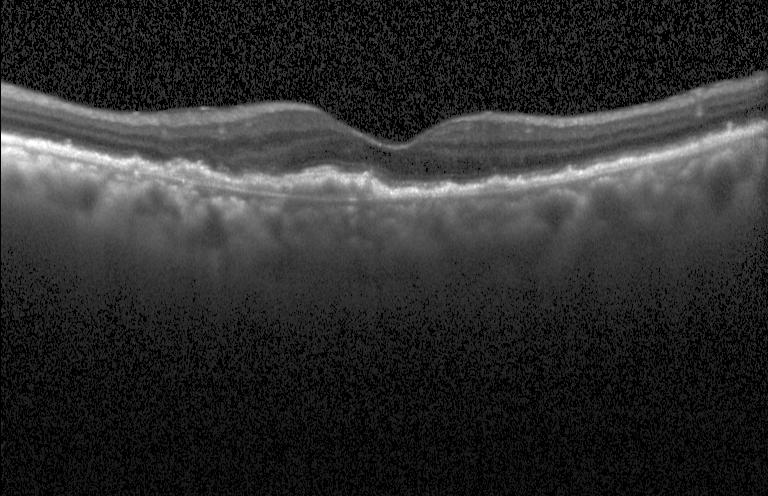
Macular OCT demonstrating a choroidal neovascular membrane.